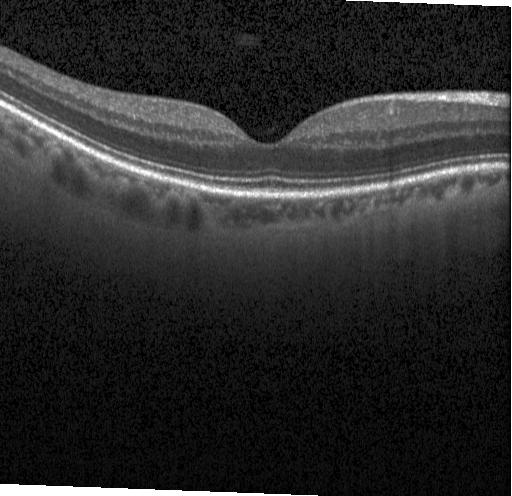

Heidelberg Spectralis. Optical coherence tomography scan.
This B-scan demonstrates no CNV, DME, or drusen.